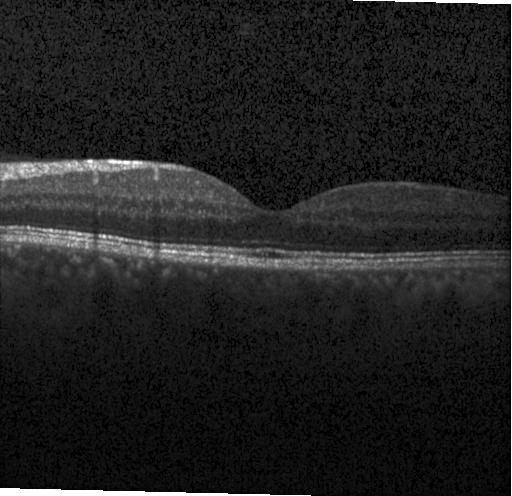

Retinal OCT cross-section showing no evidence of CNV, DME, or drusen.